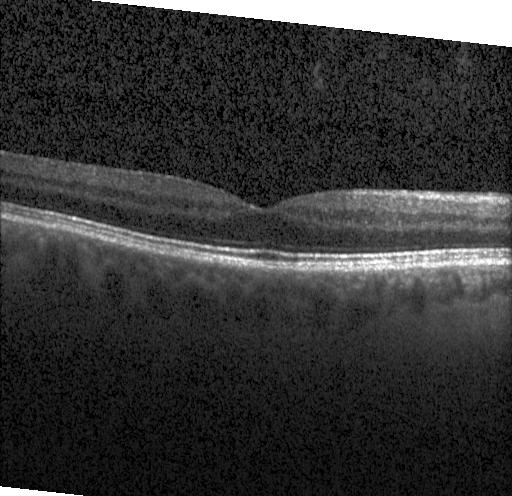
Macular OCT: no evidence of choroidal neovascularization, diabetic macular edema, or drusen.